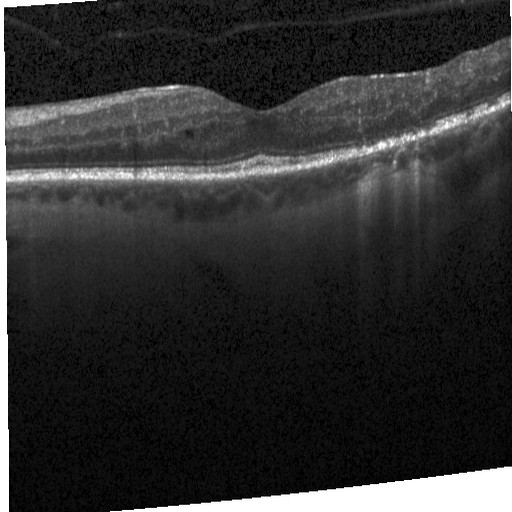
OCT line scan · centered on the fovea · Heidelberg Spectralis · spectral-domain OCT — Impression: diabetic macular edema.